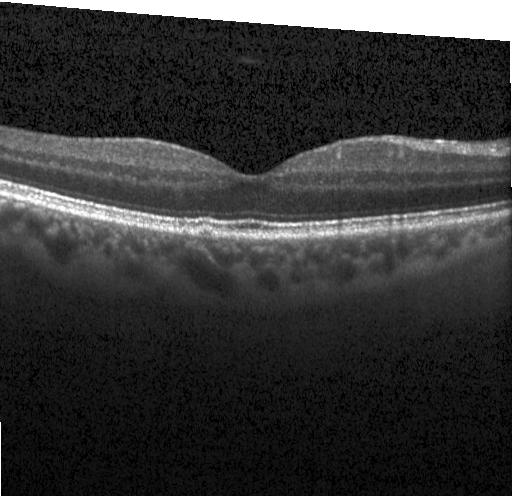 OCT B-scan, Heidelberg Spectralis OCT system, SD-OCT, centered on the fovea.
Impression: sub-RPE drusenoid deposits.